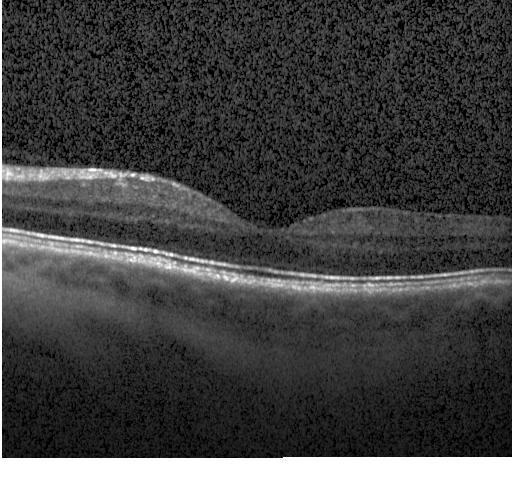
OCT B-scan showing neither choroidal neovascularization, diabetic macular edema, nor drusen.